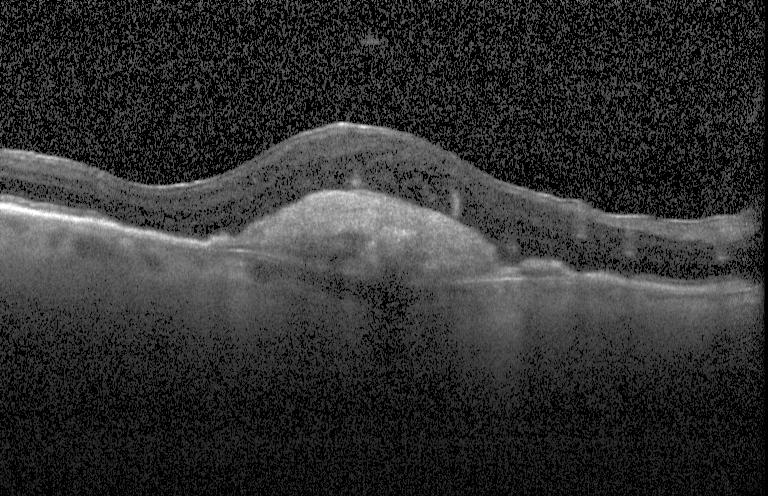

Heidelberg Spectralis. OCT line scan. Centered on the fovea. Spectral-domain OCT. The scan shows a choroidal neovascular membrane.